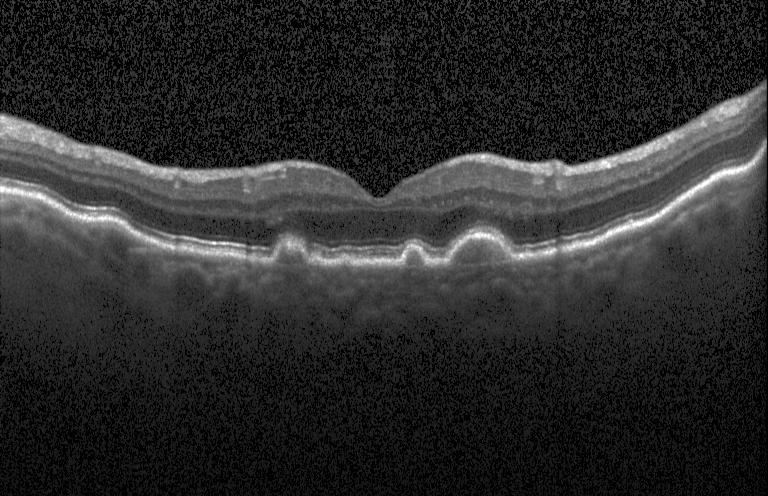

Macular OCT demonstrating drusen.